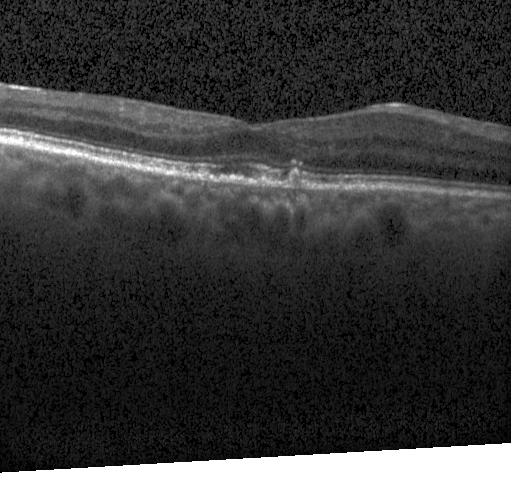

Drusen.